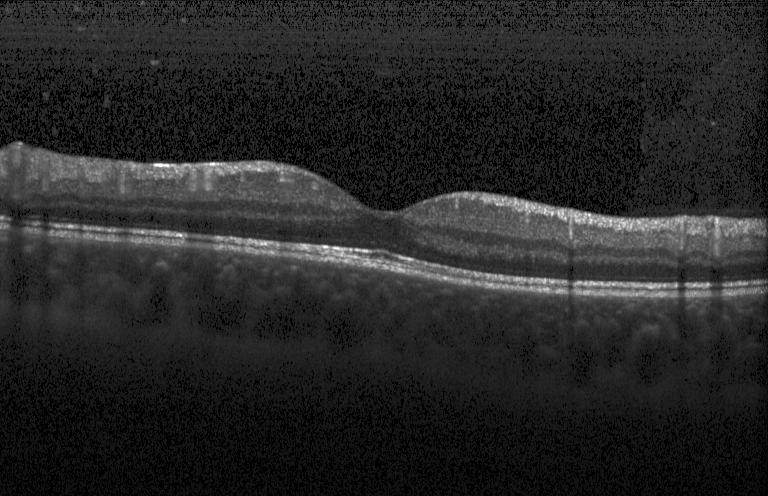 Spectral-domain OCT, OCT B-scan, macular scan — Dx: no CNV, DME, or drusen.